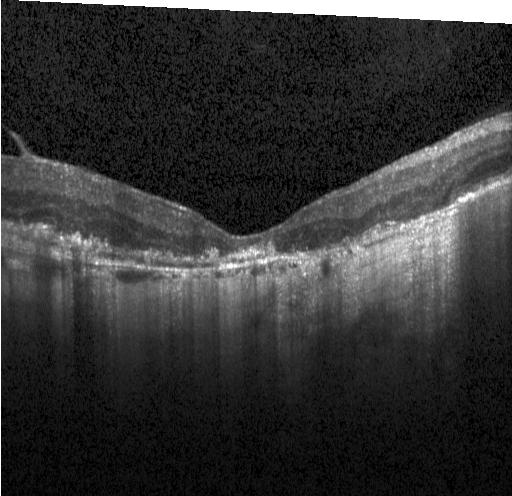
Retinal OCT B-scan.
This B-scan demonstrates choroidal neovascularization (CNV).